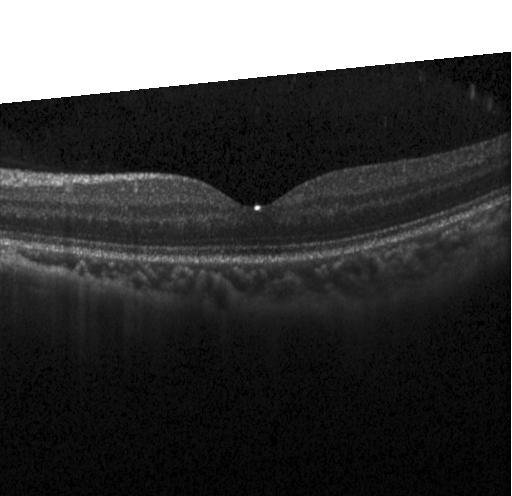 Optical coherence tomography scan · centered on the fovea. Diagnosis: no CNV, DME, or drusen.